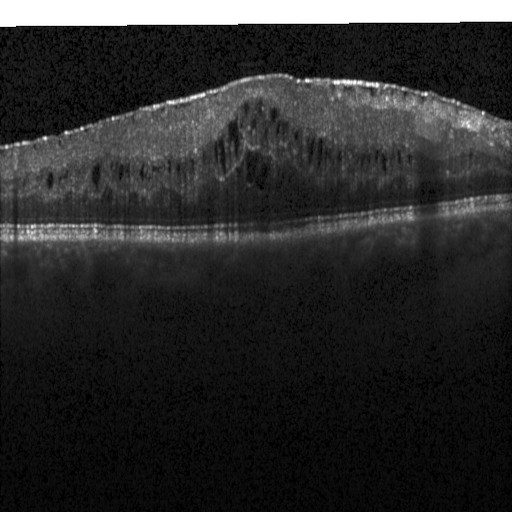

OCT B-scan. OCT finding: diabetic macular edema.